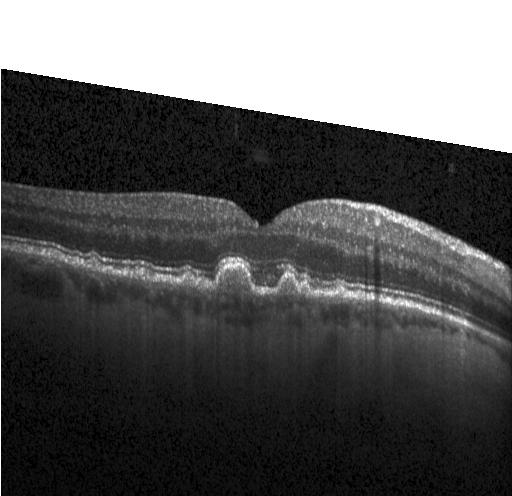 Spectral-domain OCT B-scan: multiple drusen.